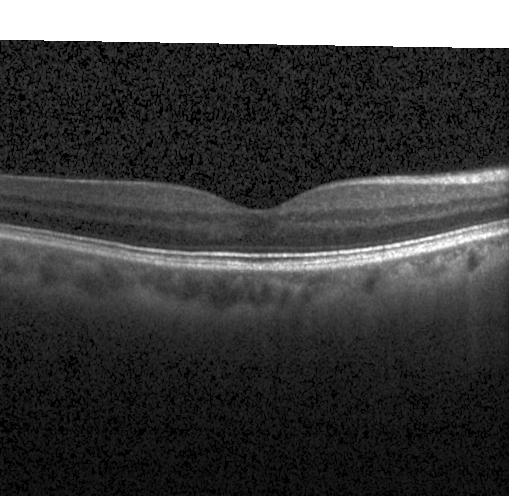

Impression: no CNV, no DME, and no drusen.